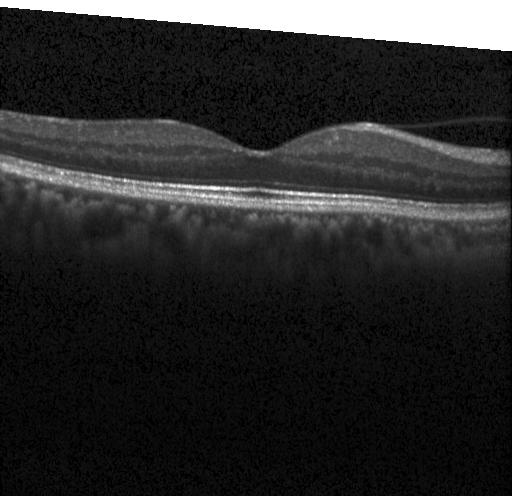 Spectral-domain optical coherence tomography, retinal OCT B-scan
No evidence of choroidal neovascularization, diabetic macular edema, or drusen.